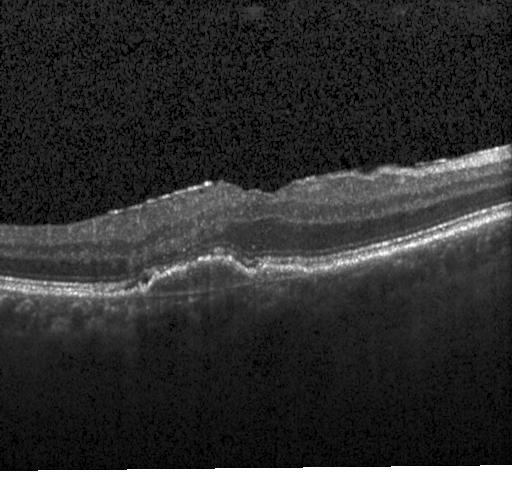
Instrument: Heidelberg Spectralis · retinal OCT B-scan · spectral-domain OCT · centered on the fovea — Finding: a choroidal neovascular membrane.